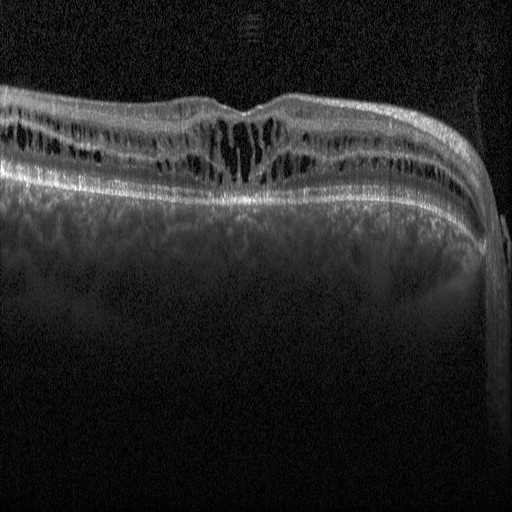 OCT scan showing diabetic macular edema (DME).